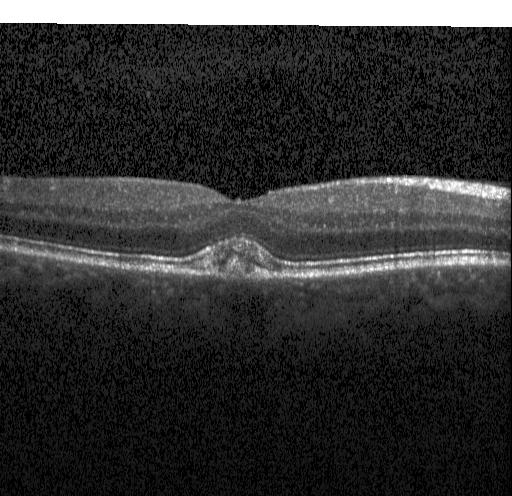 Optical coherence tomography scan · through the macula · Heidelberg Spectralis OCT system.
Impression: choroidal neovascularization (CNV).